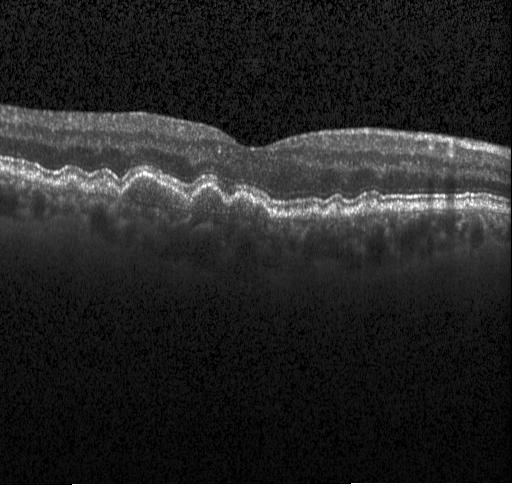
Diagnosis: multiple drusen.